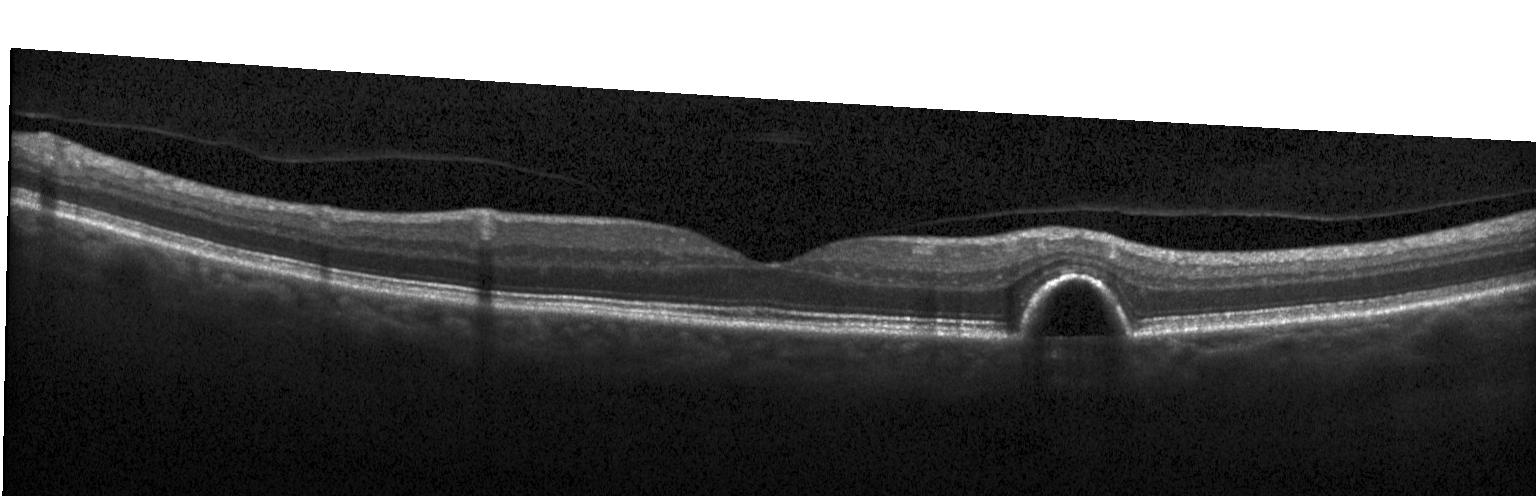 Instrument: Heidelberg Spectralis · macular scan · SD-OCT · retinal OCT cross-section
Diagnosis: choroidal neovascularization.